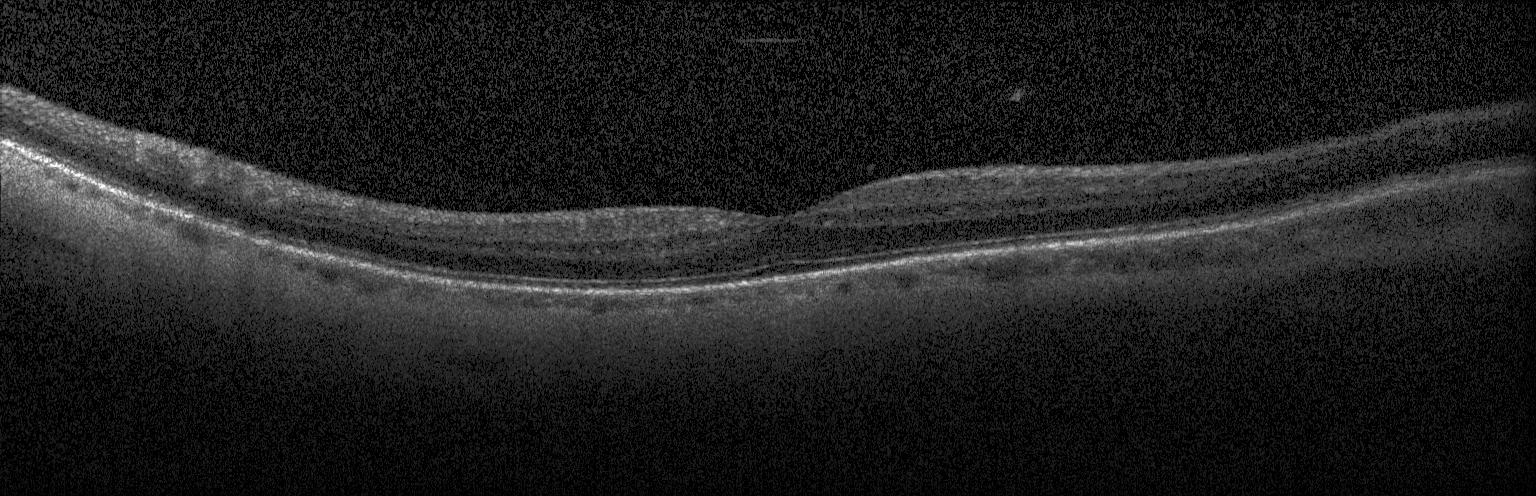
Dx: no choroidal neovascularization, diabetic macular edema, or drusen.